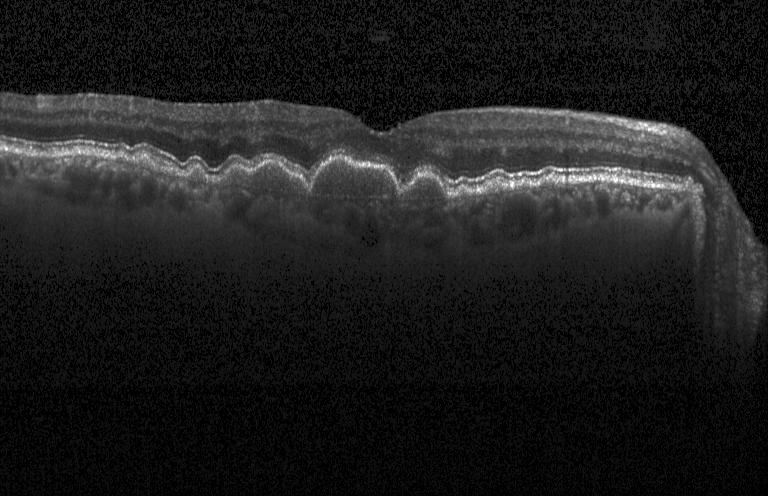

Drusen.